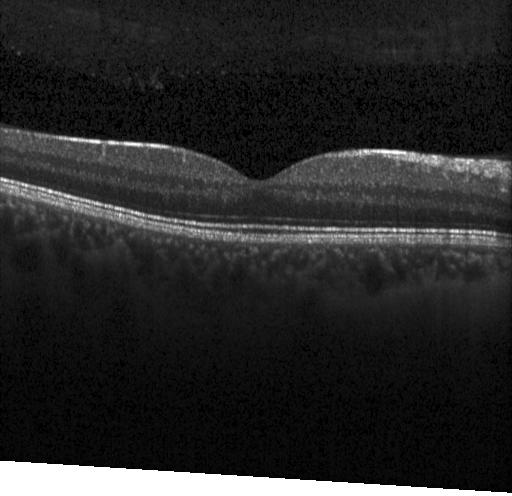
Optical coherence tomography B-scan. Fovea-centered. Diagnosis: neither CNV, DME, nor drusen.